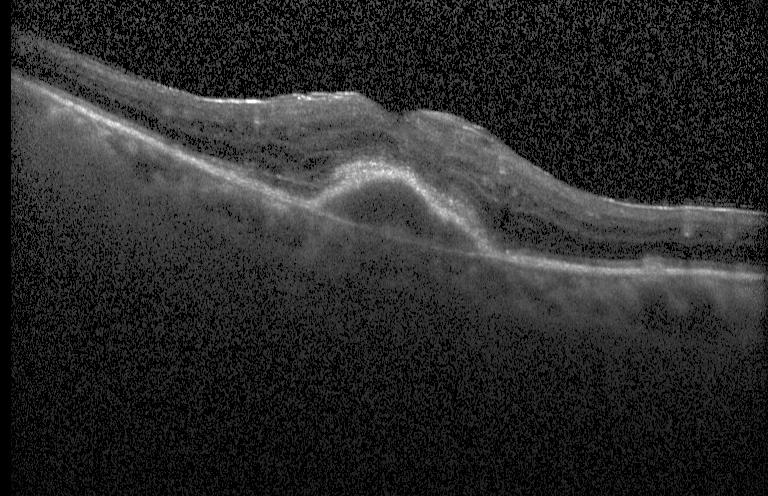
OCT finding: CNV.